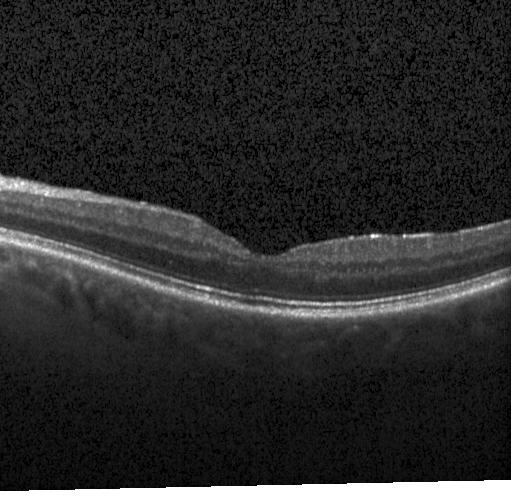

Horizontal scan through the fovea · OCT line scan.
Finding: no evidence of CNV, DME, or drusen.